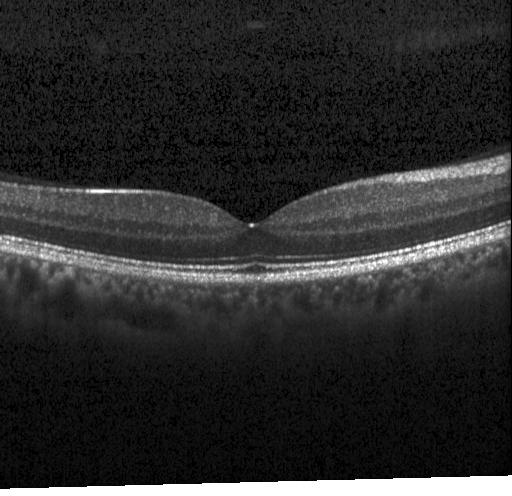
Optical coherence tomography B-scan, spectral-domain OCT
Assessment: neither choroidal neovascularization, diabetic macular edema, nor drusen.